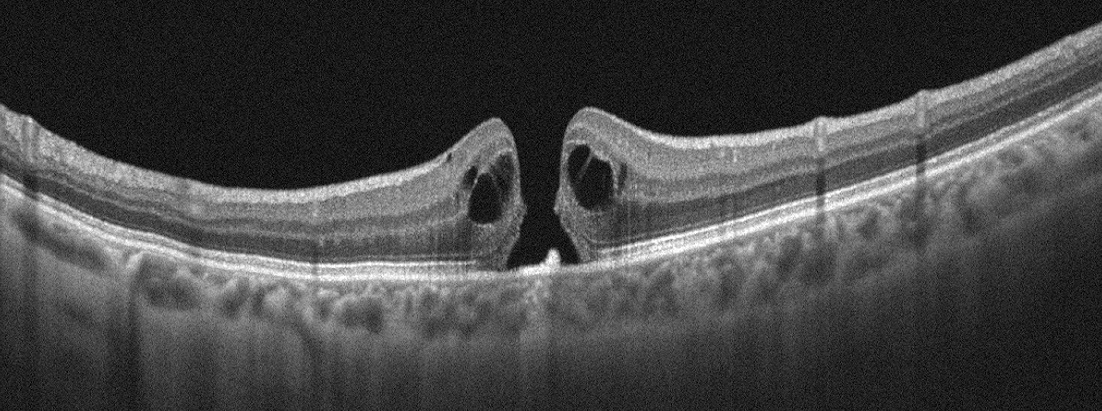
Retinal OCT B-scan. Finding: vitreomacular interface disease.